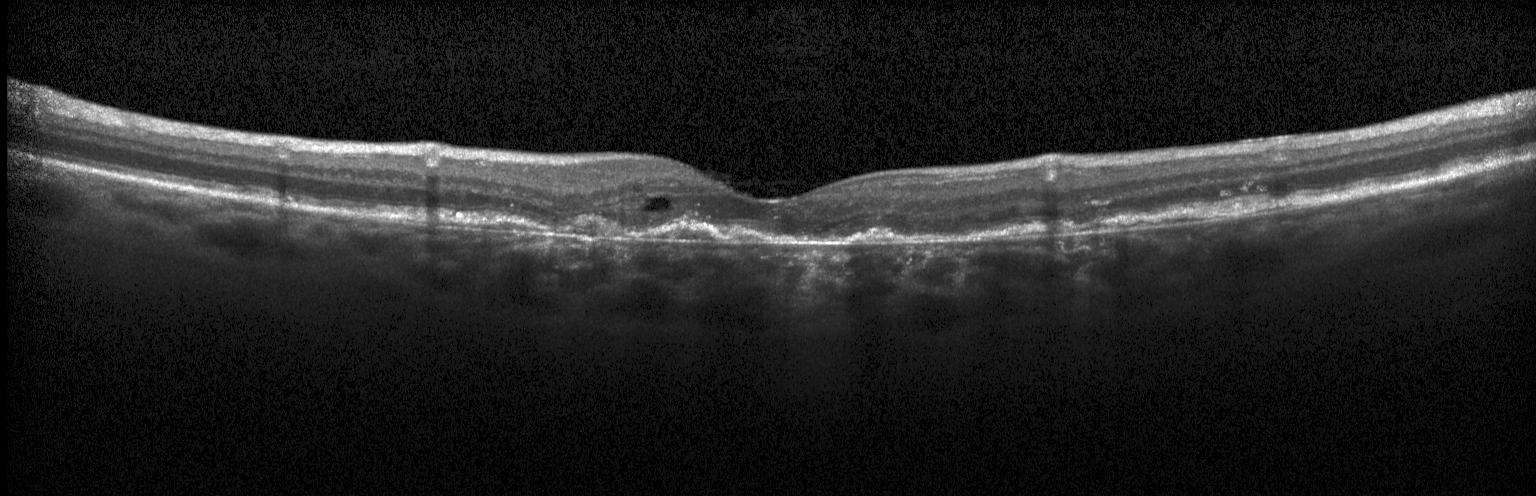 Acquired on a Heidelberg Spectralis. Retinal OCT B-scan. Macular scan. Diagnosis: a choroidal neovascular membrane.